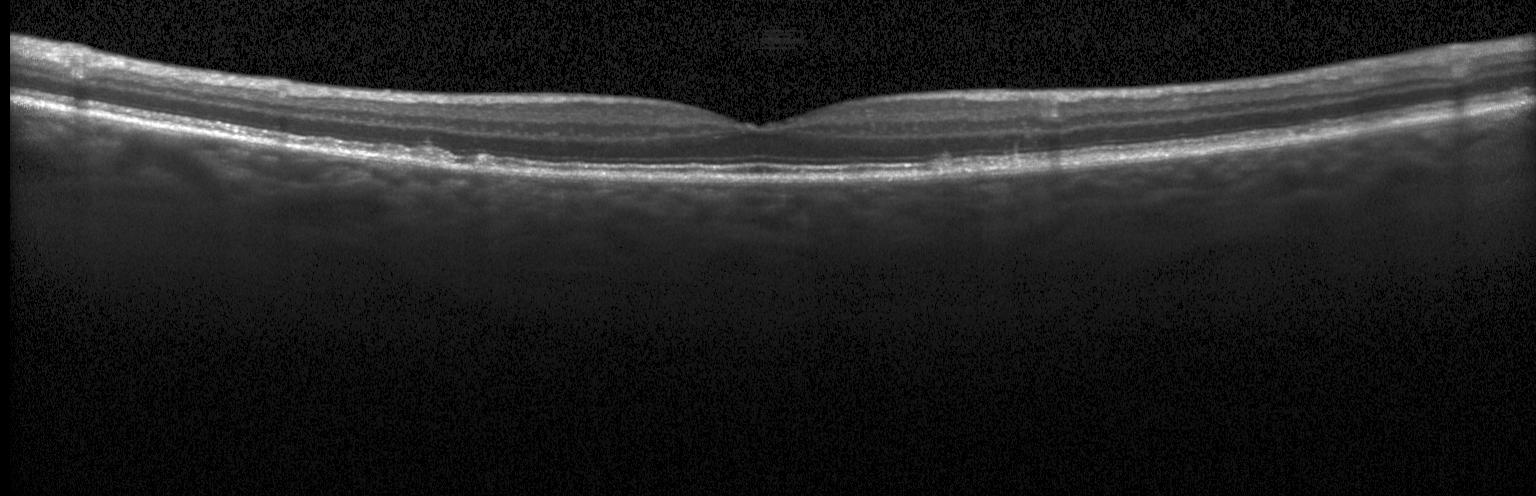
OCT line scan — Drusen.